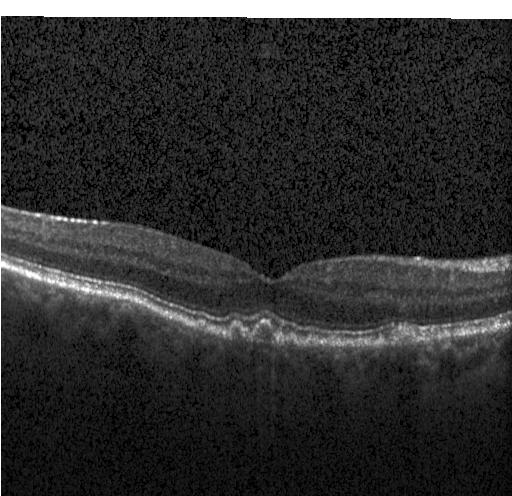
Dx: drusen.